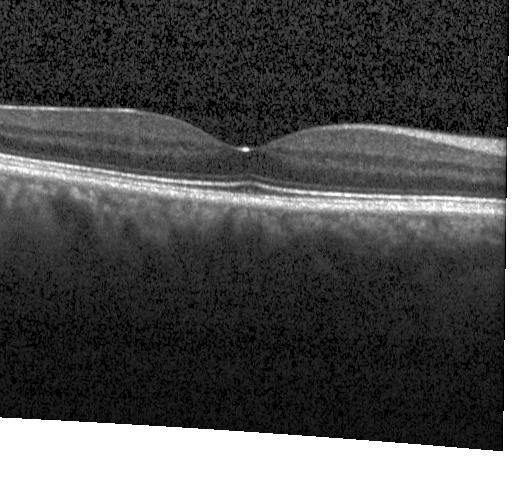

Optical coherence tomography scan. Spectral-domain OCT. Finding: no choroidal neovascularization, diabetic macular edema, or drusen.